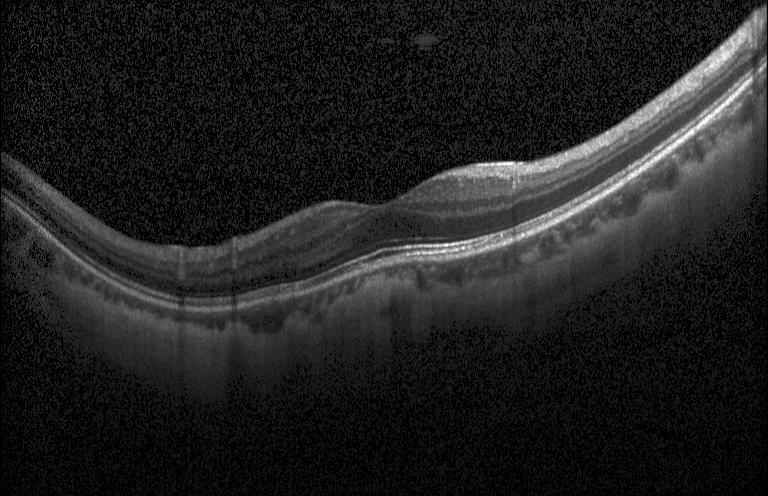 OCT B-scan, macular scan, spectral-domain OCT.
Impression: no evidence of CNV, DME, or drusen.